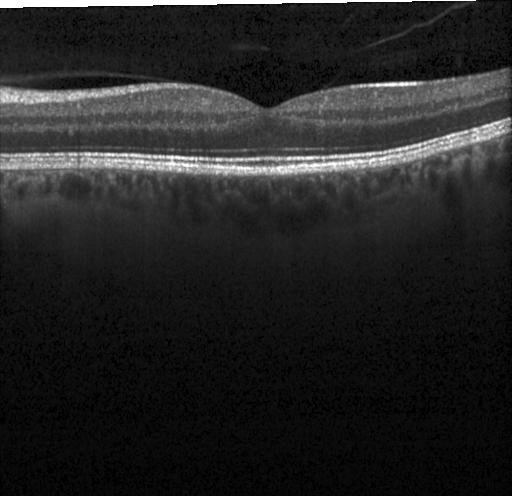 Heidelberg Spectralis, optical coherence tomography B-scan, spectral-domain OCT, fovea-centered
Impression: no evidence of CNV, DME, or drusen.